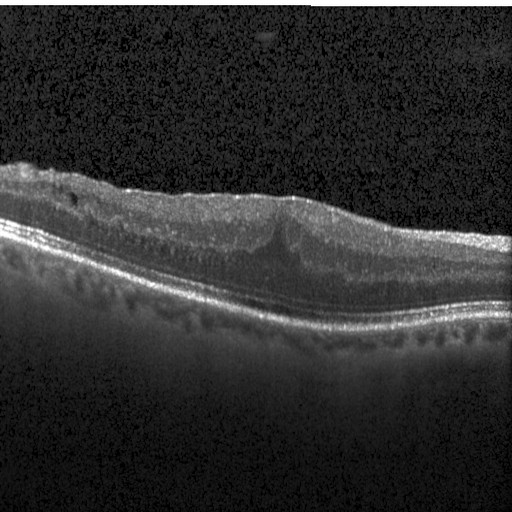
Spectral-domain OCT B-scan: diabetic macular edema.